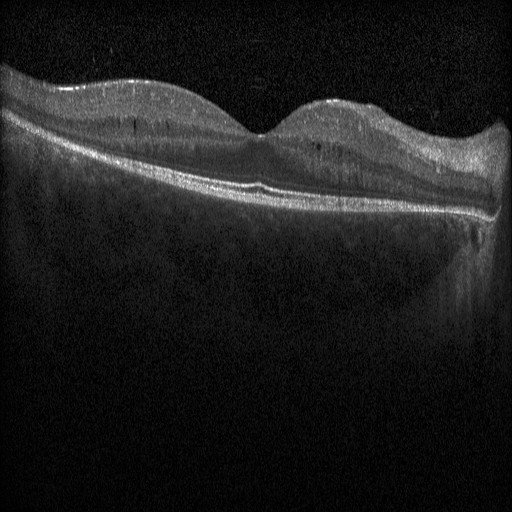
Macular OCT demonstrating diabetic macular edema.